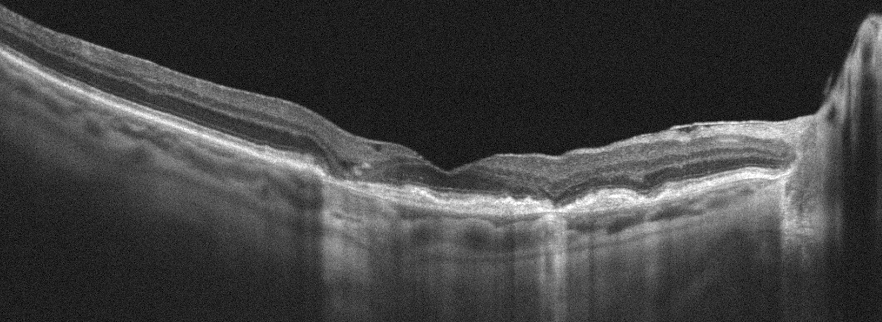 Impression: age-related macular degeneration.